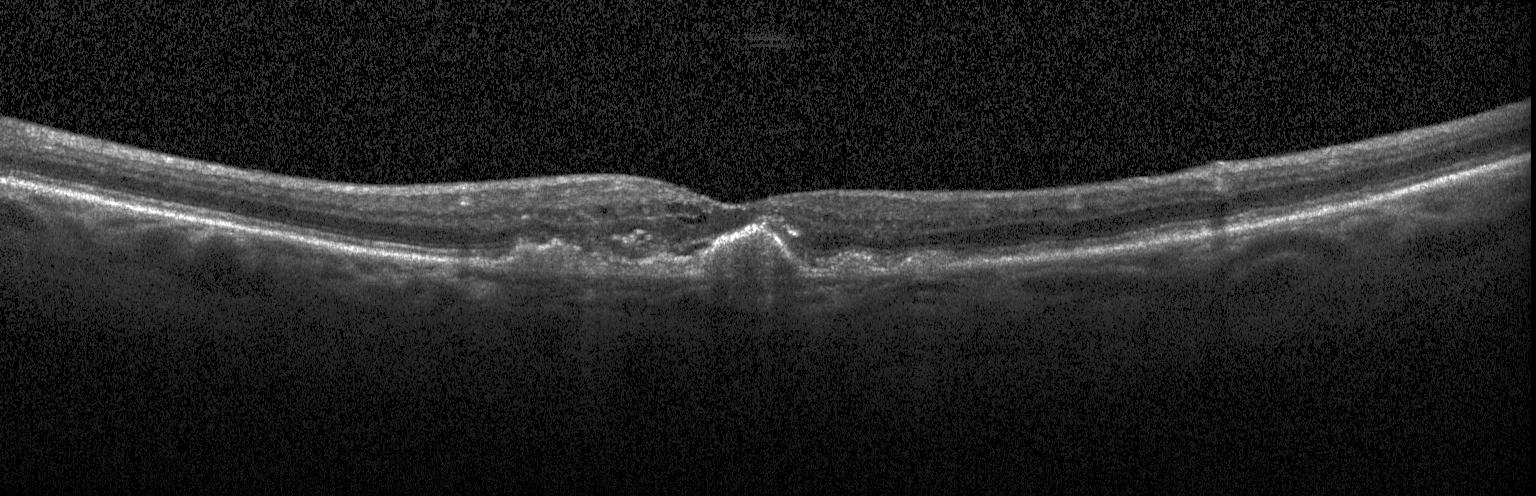 OCT B-scan showing a choroidal neovascular membrane.